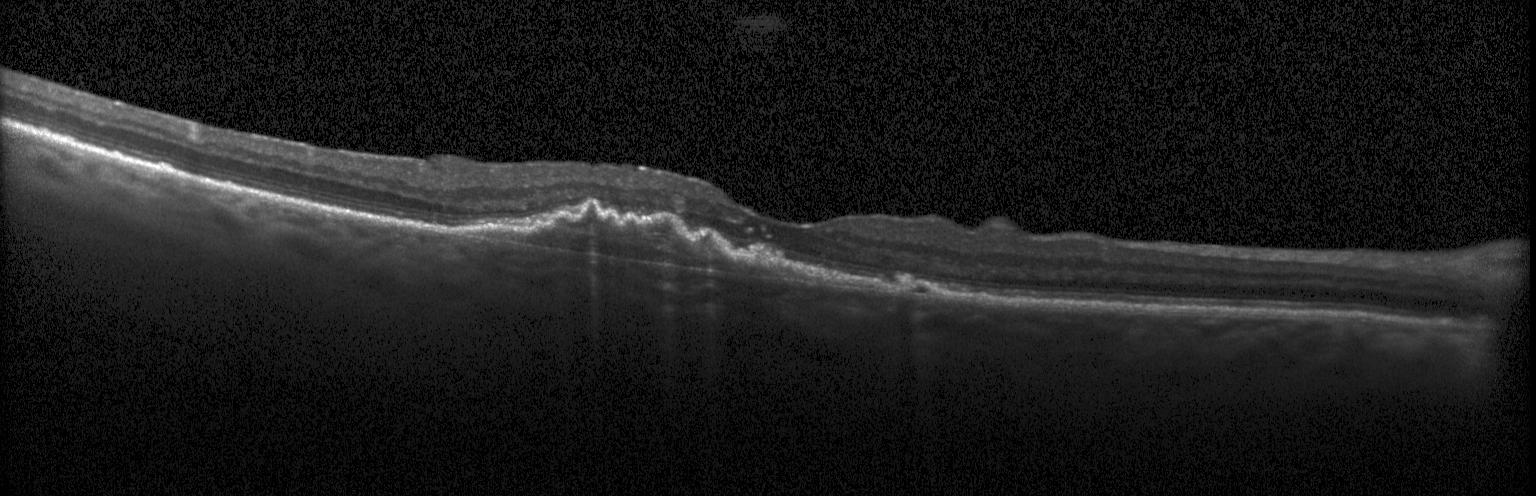
OCT finding: a choroidal neovascular membrane.